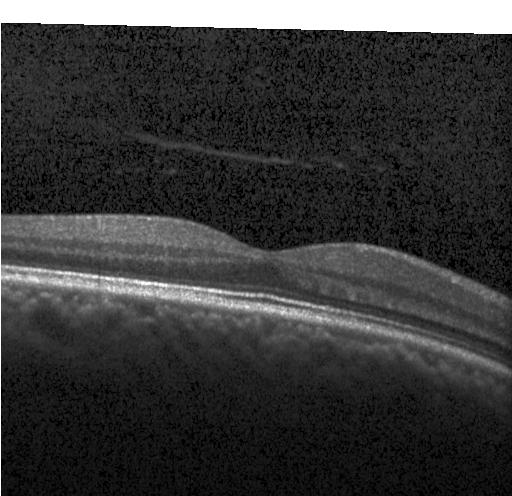

Instrument: Heidelberg Spectralis, optical coherence tomography B-scan, spectral-domain OCT
OCT finding: no evidence of choroidal neovascularization, diabetic macular edema, or drusen.